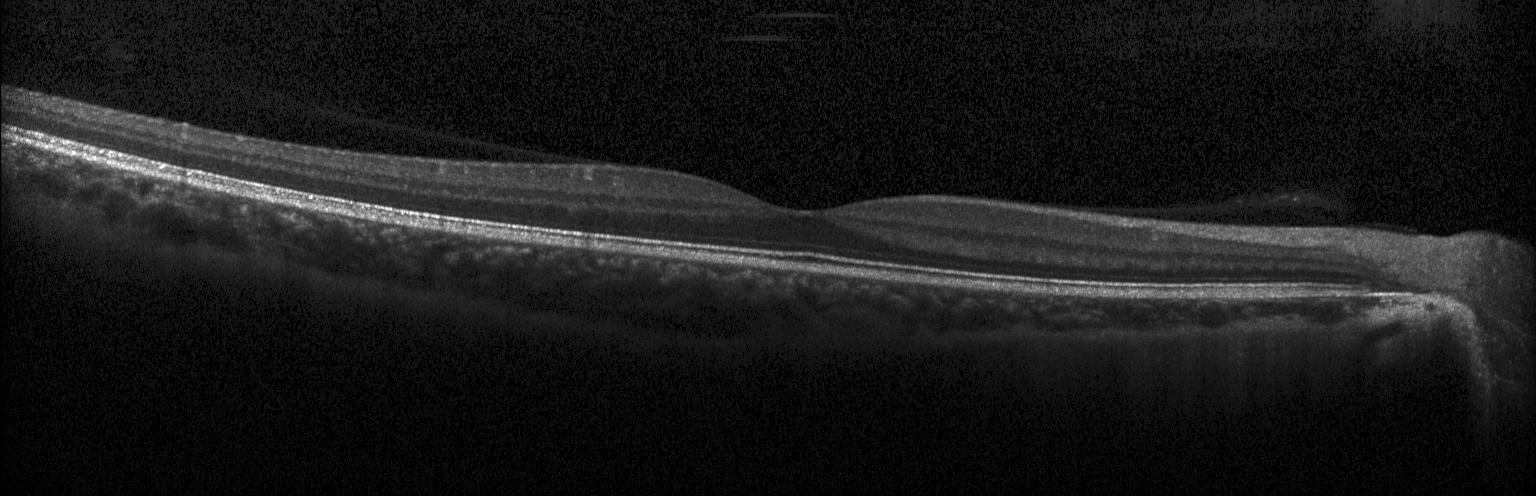
Centered on the fovea · optical coherence tomography scan · spectral-domain OCT · acquired on a Heidelberg Spectralis — Impression: no evidence of choroidal neovascularization, diabetic macular edema, or drusen.